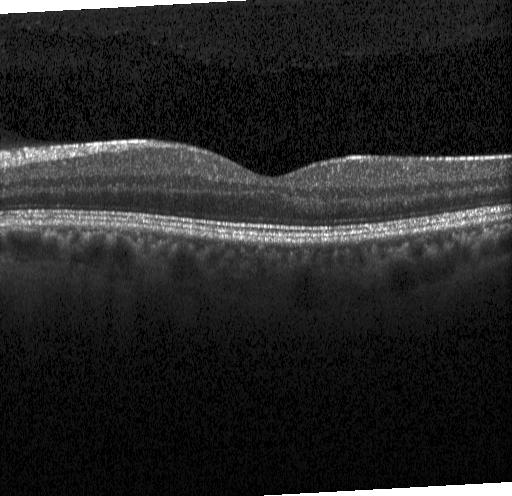
Spectral-domain optical coherence tomography, OCT line scan, acquired on a Heidelberg Spectralis, centered on the fovea — The scan shows no evidence of CNV, DME, or drusen.